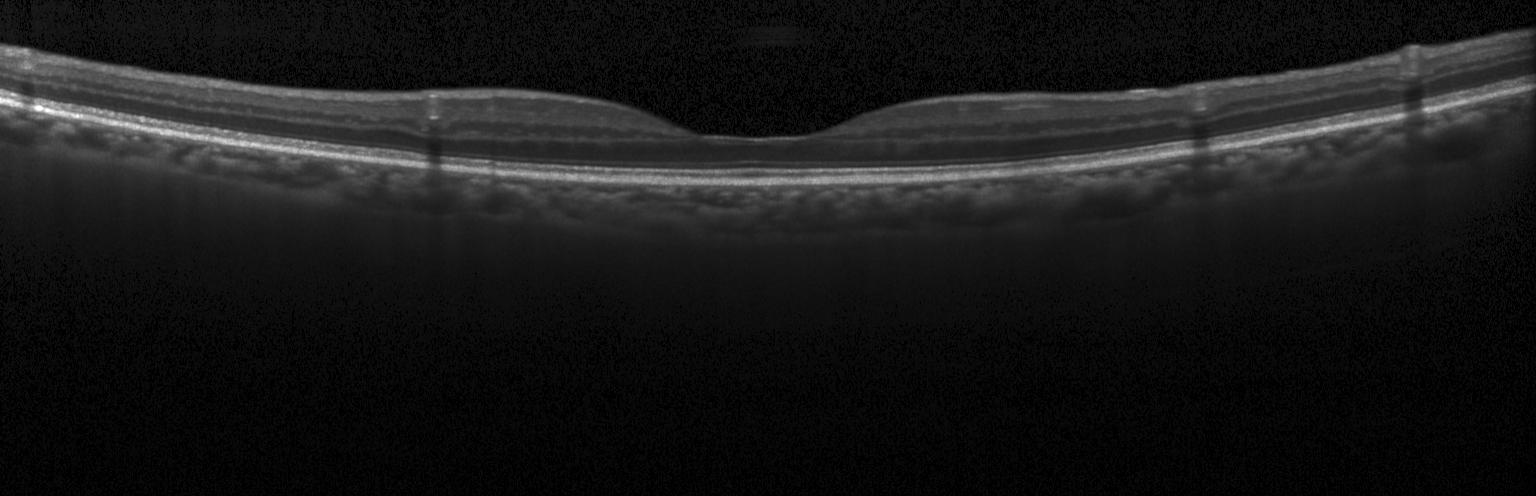

Centered on the fovea · spectral-domain optical coherence tomography · Heidelberg Spectralis OCT system · optical coherence tomography B-scan
Diagnosis: neither choroidal neovascularization, diabetic macular edema, nor drusen.